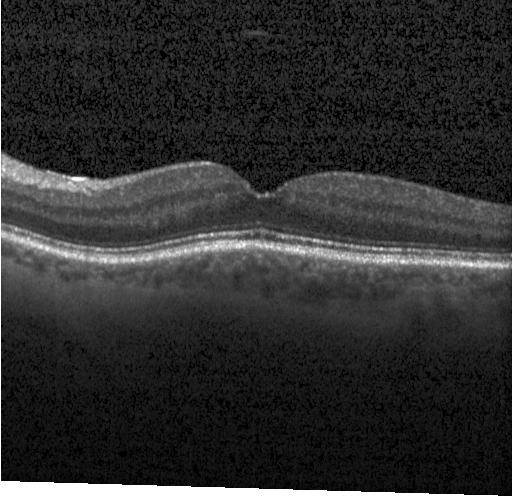

OCT B-scan · SD-OCT · Heidelberg Spectralis · macular scan.
No CNV, DME, or drusen.